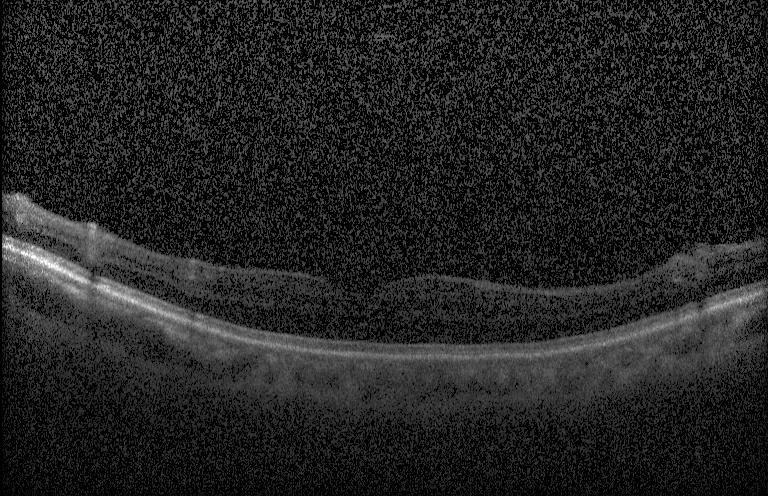
OCT scan showing no choroidal neovascularization, no diabetic macular edema, and no drusen.